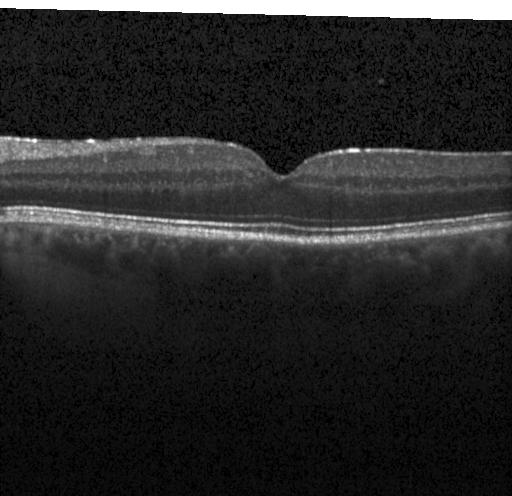

SD-OCT. OCT B-scan. Finding: no evidence of choroidal neovascularization, diabetic macular edema, or drusen.